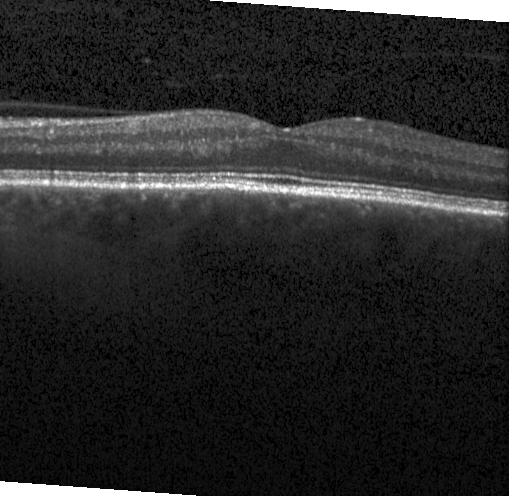 Acquired on a Heidelberg Spectralis. Retinal OCT B-scan.
Diagnosis: no evidence of choroidal neovascularization, diabetic macular edema, or drusen.